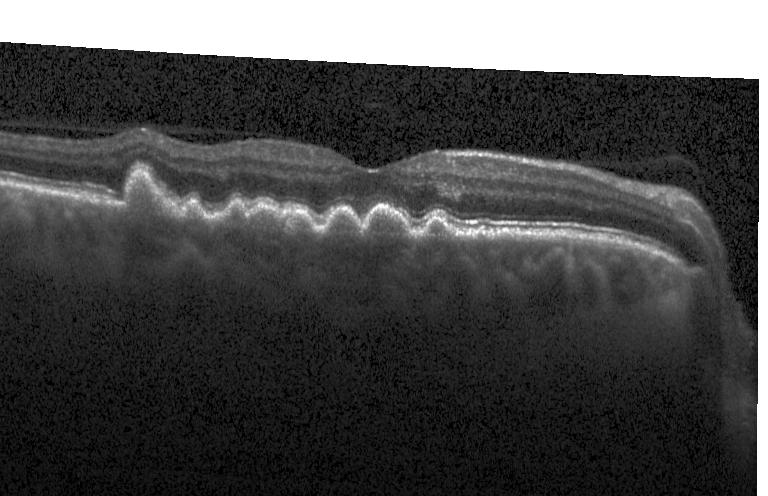

Retinal OCT cross-section showing sub-RPE drusenoid deposits.